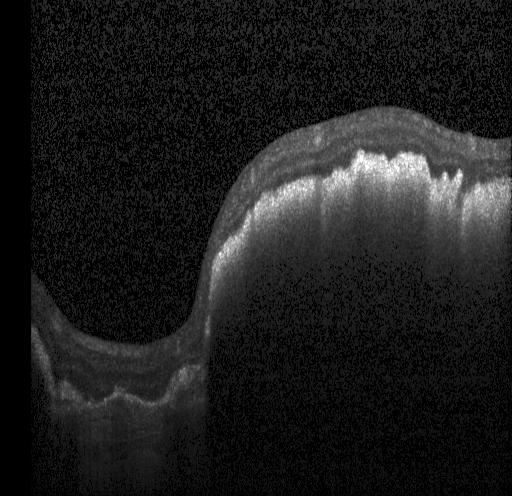 Retinal OCT cross-section — The scan shows a choroidal neovascular membrane.